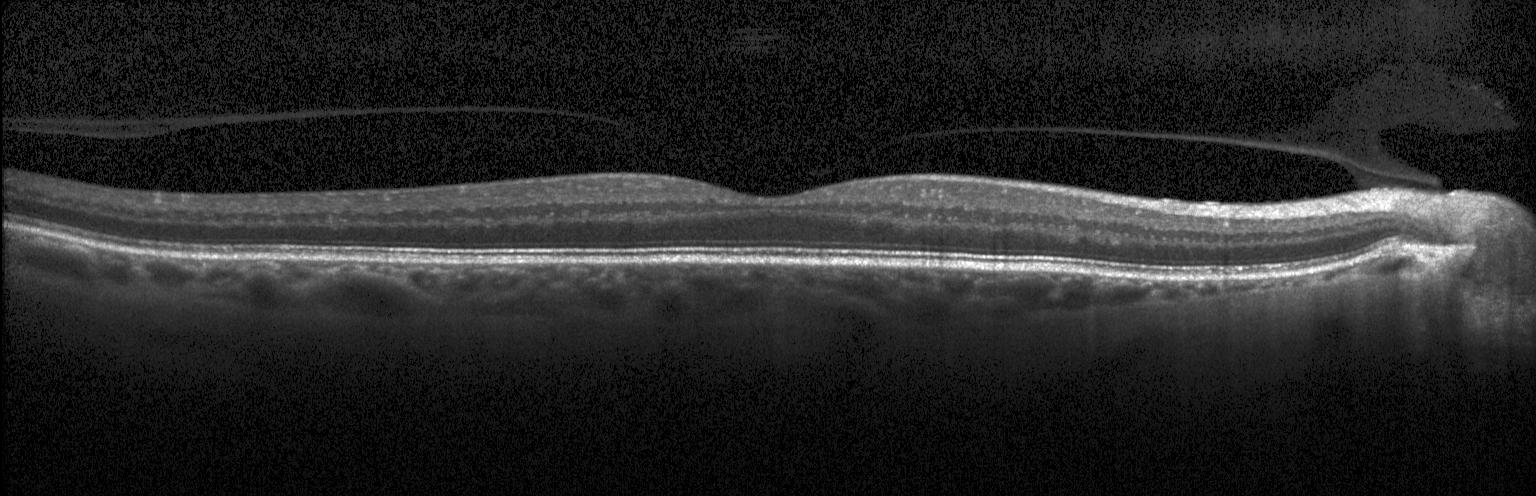

No choroidal neovascularization, diabetic macular edema, or drusen.